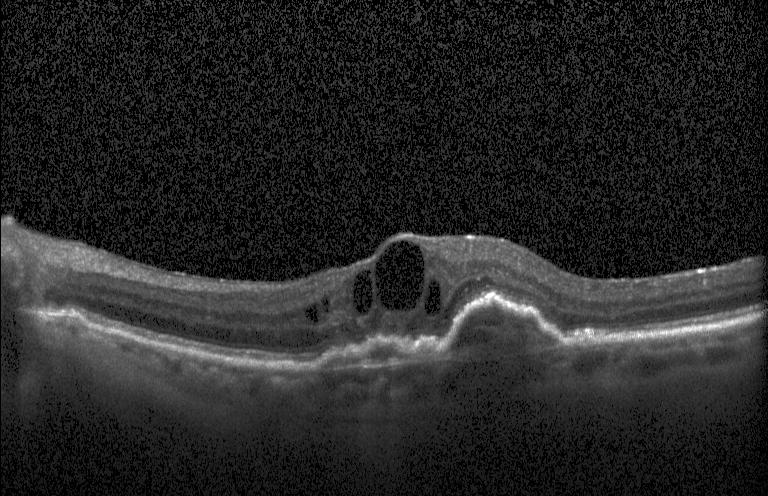
Diagnosis: a choroidal neovascular membrane.